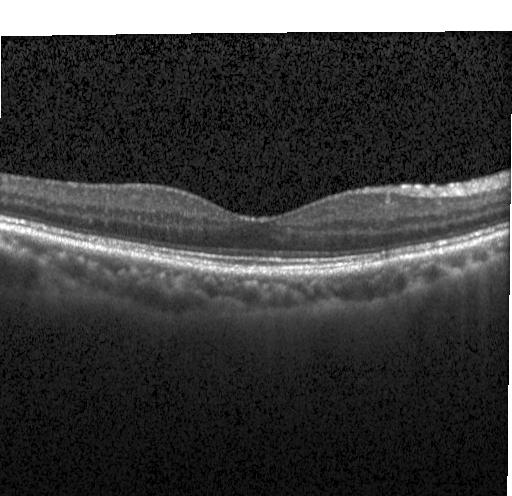
Finding: neither choroidal neovascularization, diabetic macular edema, nor drusen.